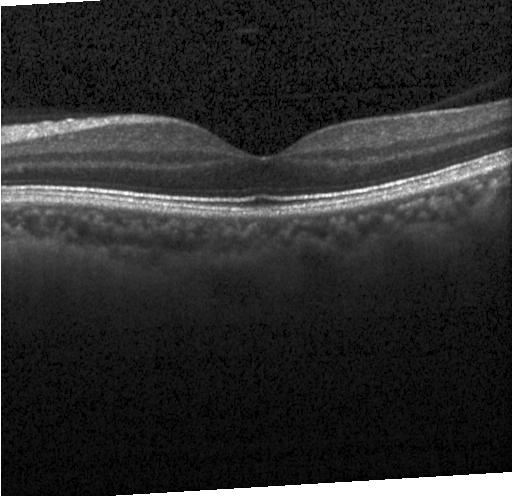
OCT B-scan
Dx: no choroidal neovascularization, diabetic macular edema, or drusen.